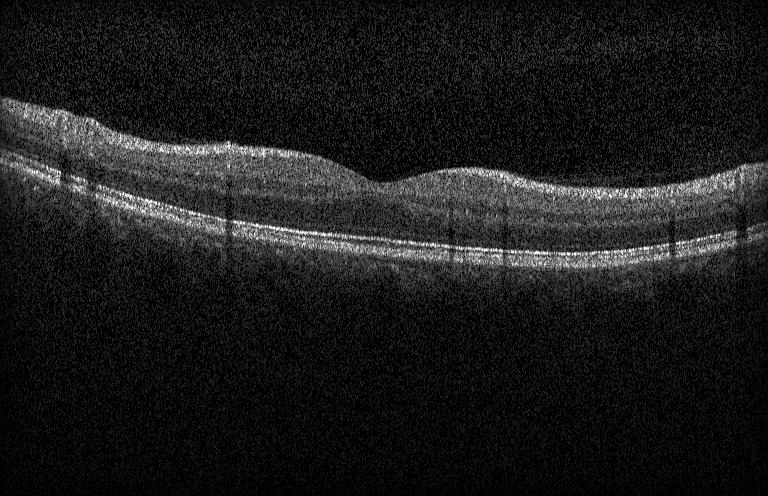

Diagnosis: neither choroidal neovascularization, diabetic macular edema, nor drusen.